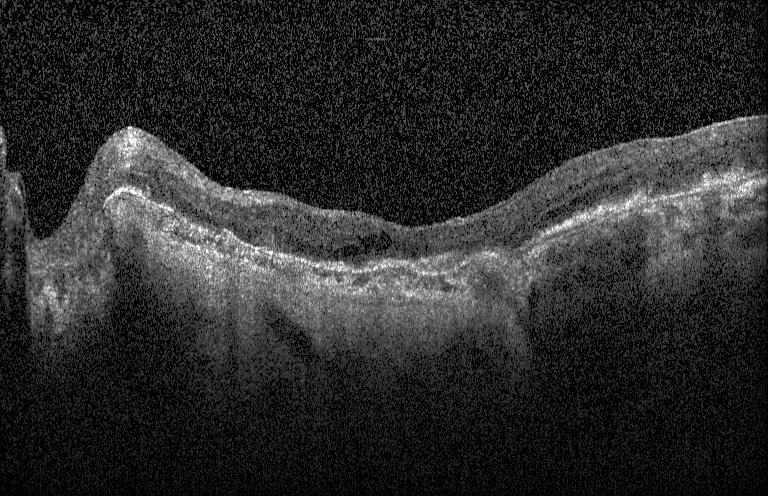
Heidelberg Spectralis · SD-OCT · retinal OCT B-scan. Diagnosis: a choroidal neovascular membrane.